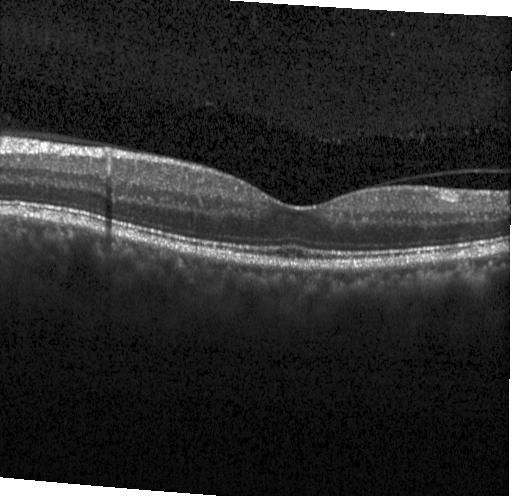 Acquired on a Heidelberg Spectralis · spectral-domain OCT · horizontal scan through the fovea · retinal OCT B-scan.
OCT finding: no evidence of choroidal neovascularization, diabetic macular edema, or drusen.